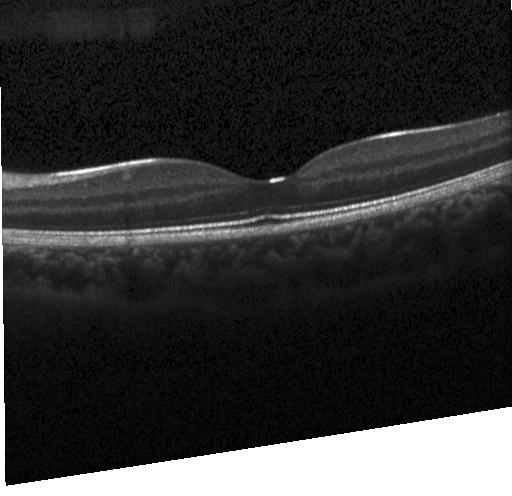

Optical coherence tomography scan.
Diagnosis: neither CNV, DME, nor drusen.